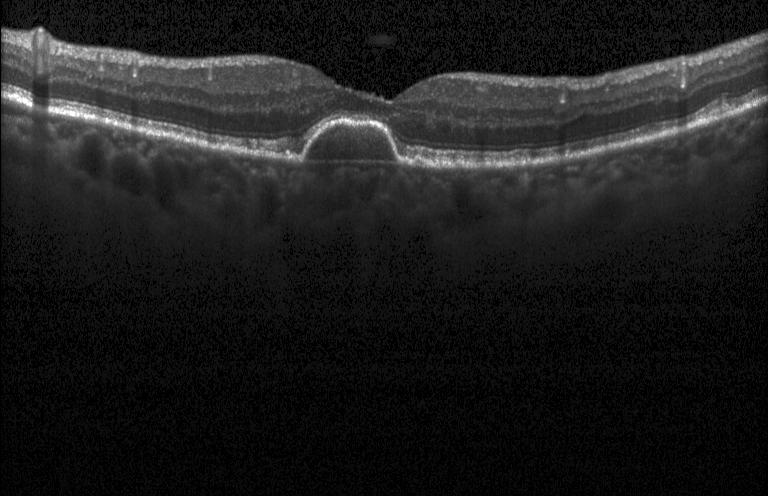 Spectral-domain OCT. Optical coherence tomography scan.
This B-scan demonstrates a choroidal neovascular membrane.